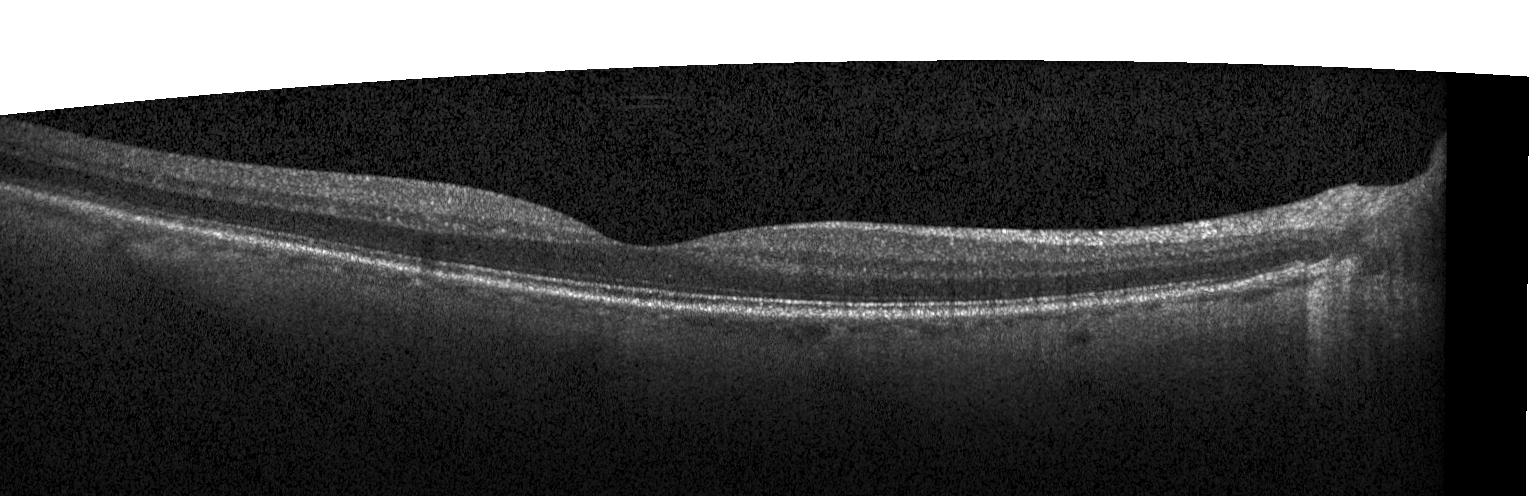 No evidence of choroidal neovascularization, diabetic macular edema, or drusen.